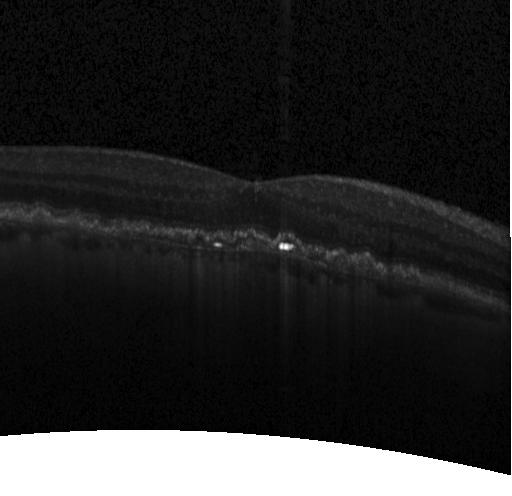
Spectral-domain OCT. Instrument: Heidelberg Spectralis. Through the macula. Optical coherence tomography B-scan.
Diagnosis: a choroidal neovascular membrane.